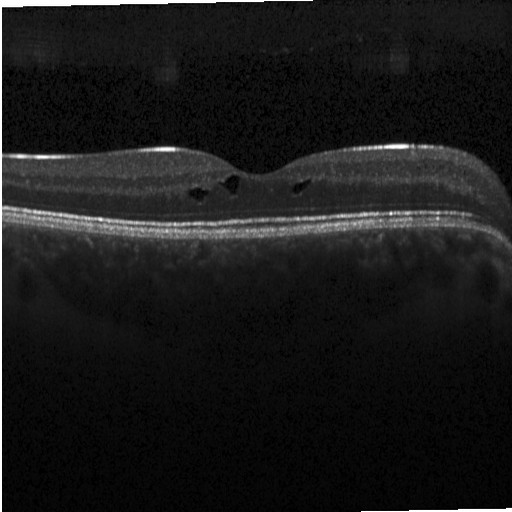 OCT B-scan. Macular scan. DME.